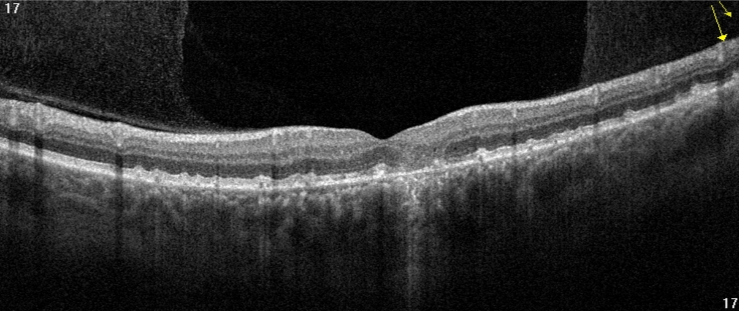
Optical coherence tomography B-scan — Diagnosis: AMD.